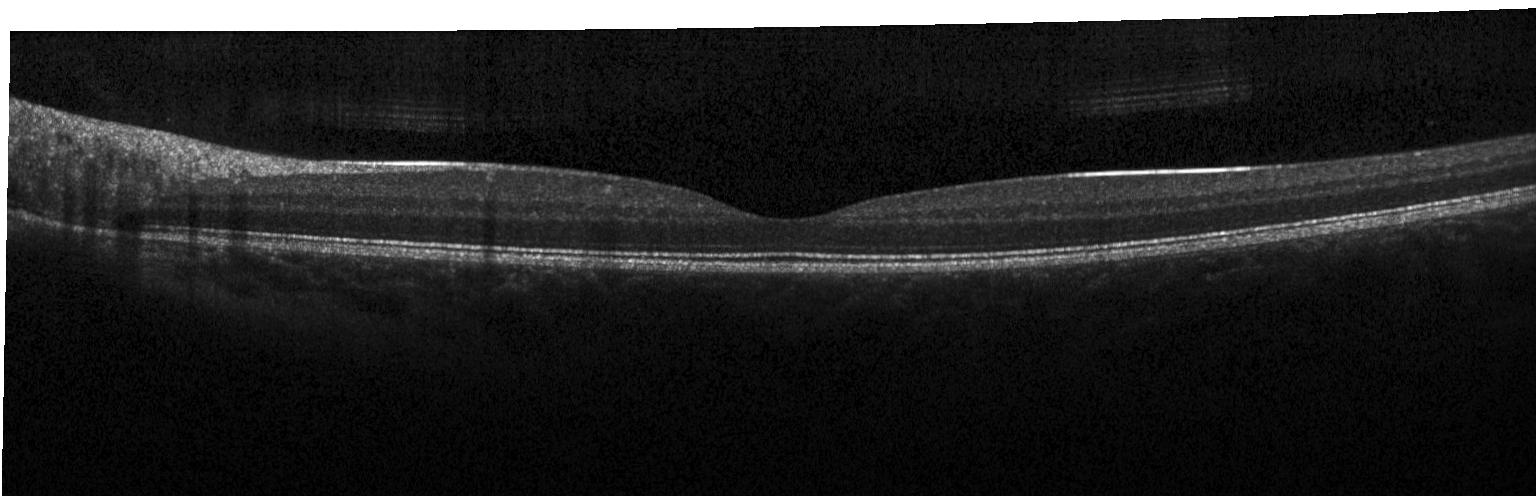
Spectral-domain OCT B-scan: no CNV, no DME, and no drusen.